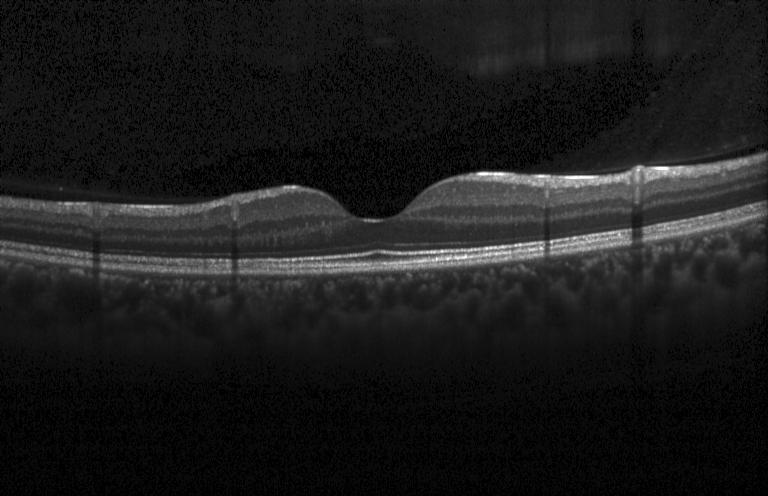
OCT B-scan. Diagnosis: no CNV, no DME, and no drusen.